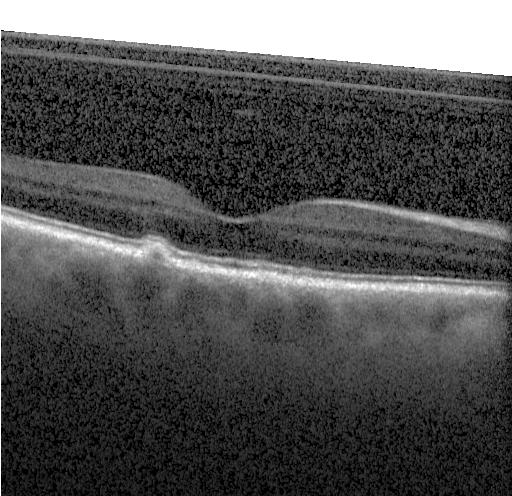 Acquired on a Heidelberg Spectralis · spectral-domain OCT · fovea-centered · optical coherence tomography scan.
This B-scan demonstrates drusen.